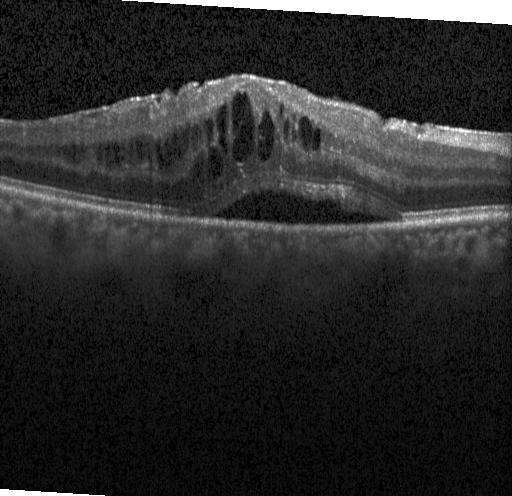

Spectral-domain OCT B-scan: diabetic macular edema (DME).